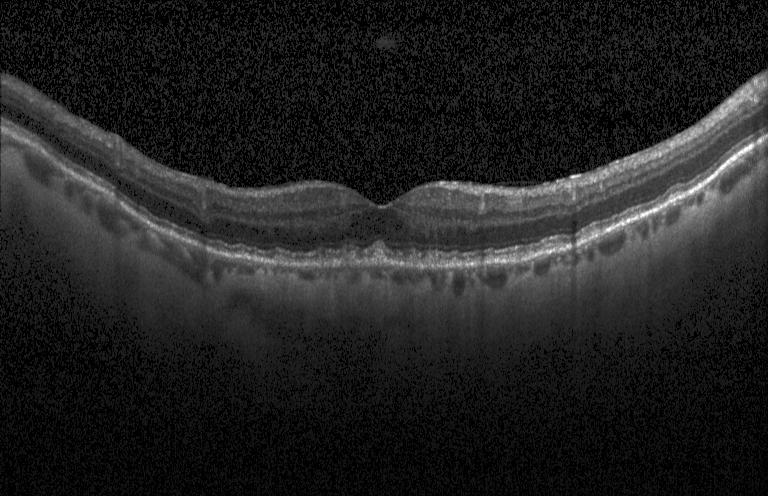 Retinal OCT B-scan. Acquired on a Heidelberg Spectralis. Through the macula. Spectral-domain optical coherence tomography.
Multiple drusen.